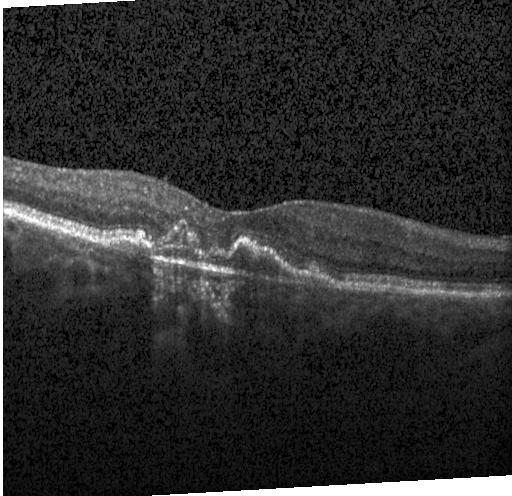
Macular OCT: a choroidal neovascular membrane.